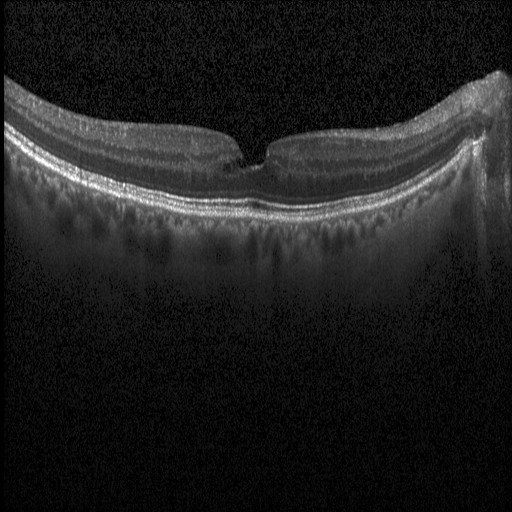
Spectral-domain OCT B-scan: diabetic macular edema (DME).